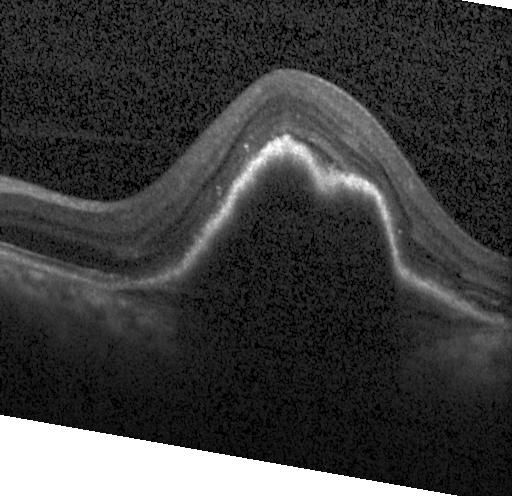
Retinal OCT B-scan · SD-OCT.
Finding: a choroidal neovascular membrane.